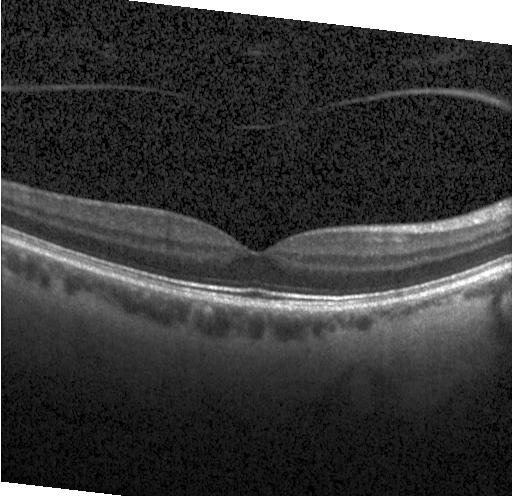

No choroidal neovascularization, no diabetic macular edema, and no drusen.